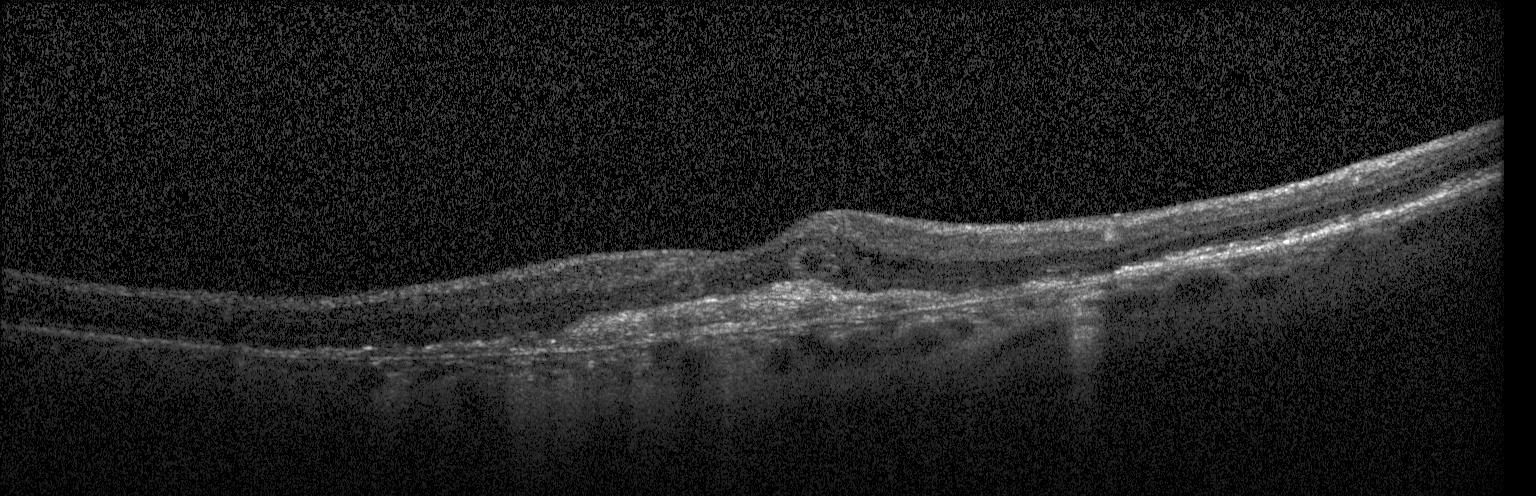

Macular scan; OCT B-scan; instrument: Heidelberg Spectralis; spectral-domain OCT
Diagnosis: a choroidal neovascular membrane.